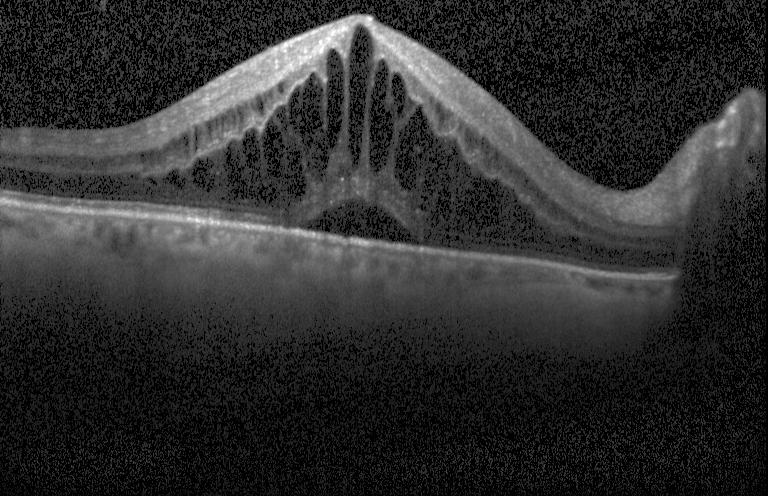

Optical coherence tomography B-scan; Heidelberg Spectralis
Finding: DME.